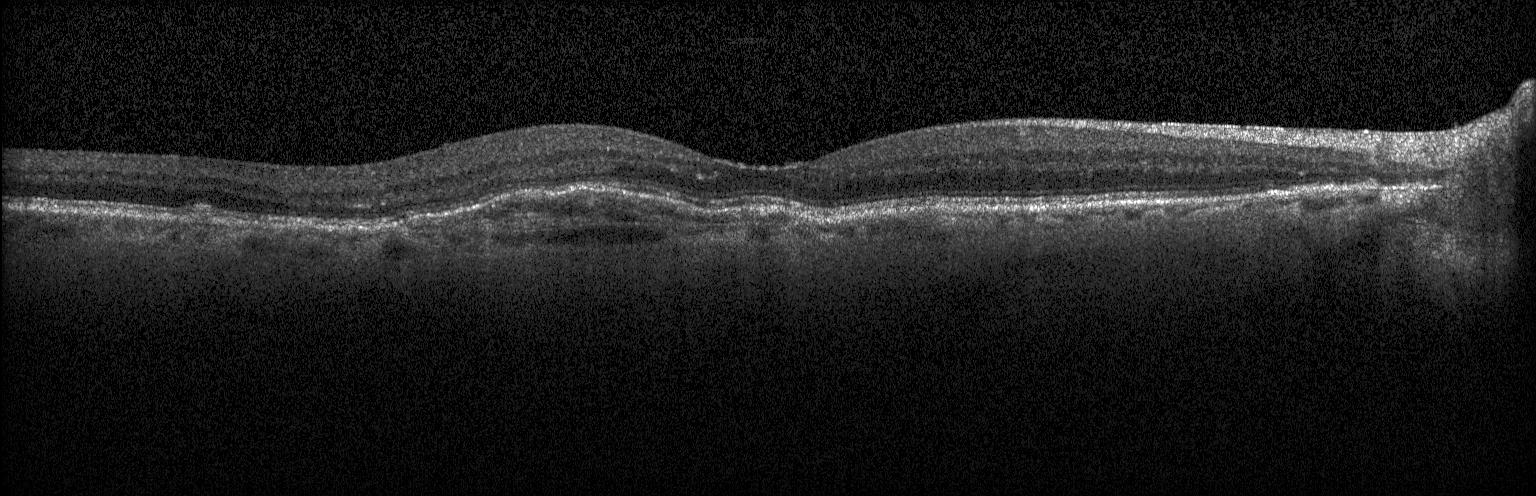
Finding: choroidal neovascularization.